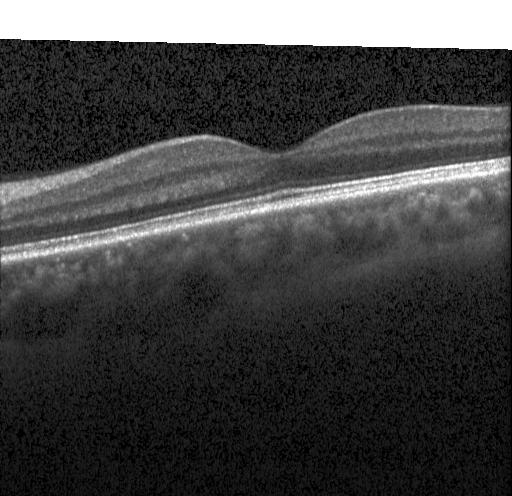

OCT B-scan; Heidelberg Spectralis OCT system — Diagnosis: neither CNV, DME, nor drusen.